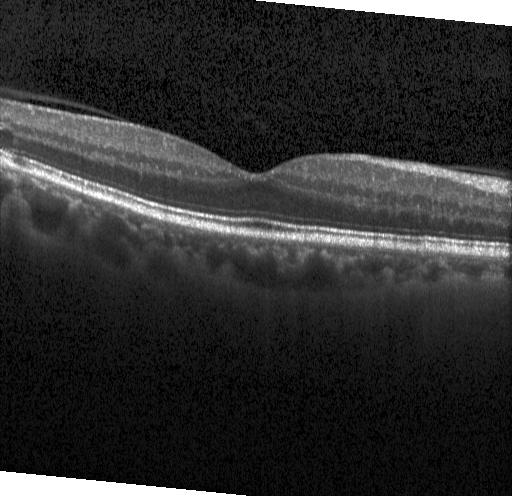
Dx: no choroidal neovascularization, no diabetic macular edema, and no drusen.